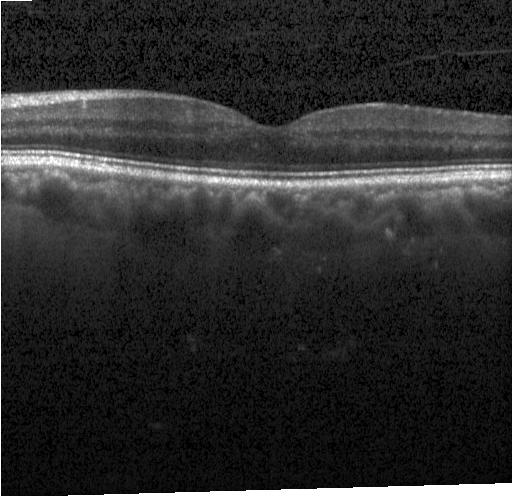 Optical coherence tomography B-scan, spectral-domain optical coherence tomography
OCT finding: no evidence of choroidal neovascularization, diabetic macular edema, or drusen.